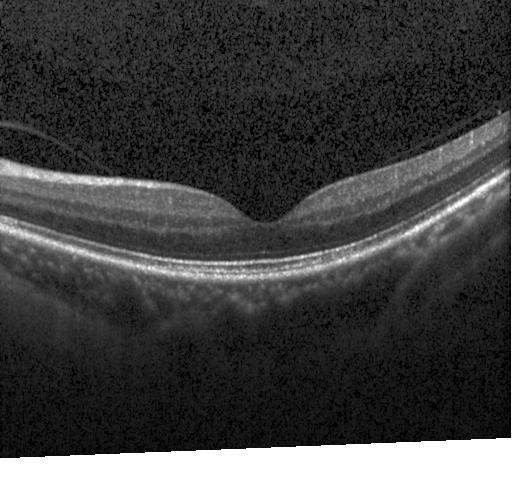
Diagnosis: no CNV, DME, or drusen.